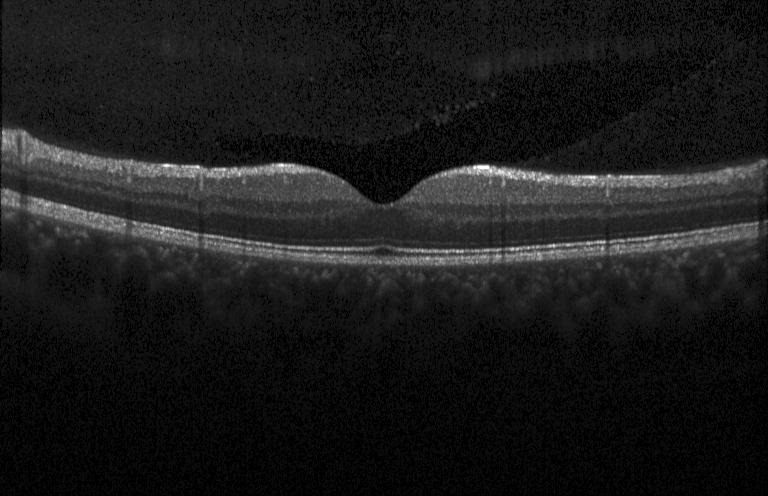
Assessment: neither choroidal neovascularization, diabetic macular edema, nor drusen.